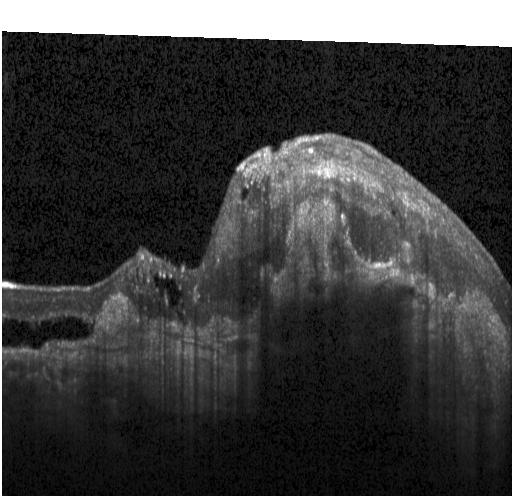
OCT B-scan · spectral-domain optical coherence tomography
Macular OCT: a choroidal neovascular membrane.